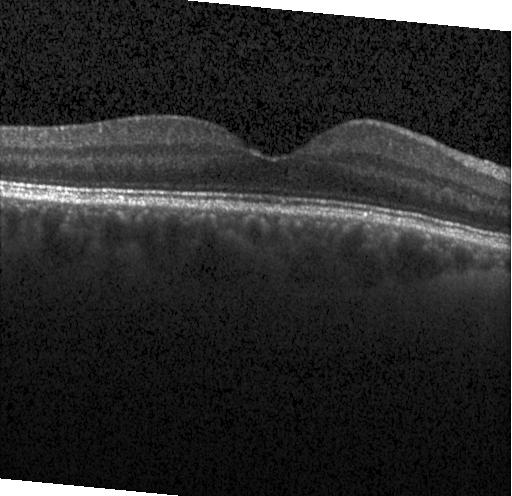

SD-OCT; centered on the fovea; acquired on a Heidelberg Spectralis; optical coherence tomography B-scan
OCT finding: no evidence of CNV, DME, or drusen.